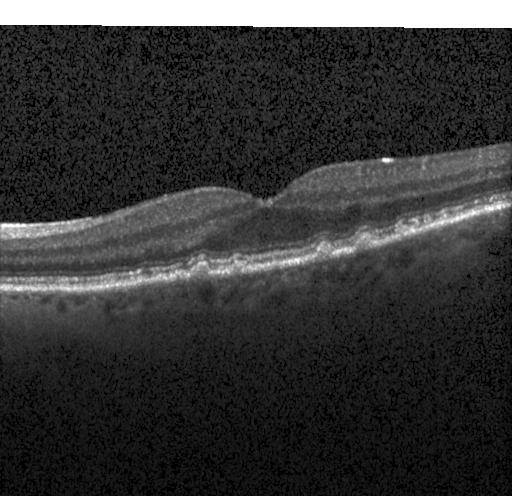
Retinal OCT cross-section, Heidelberg Spectralis OCT system, spectral-domain optical coherence tomography, through the macula.
Sub-RPE drusenoid deposits.